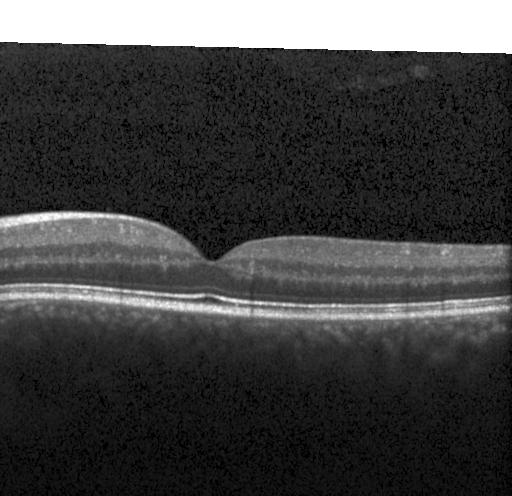 Retinal OCT cross-section — Assessment: neither CNV, DME, nor drusen.